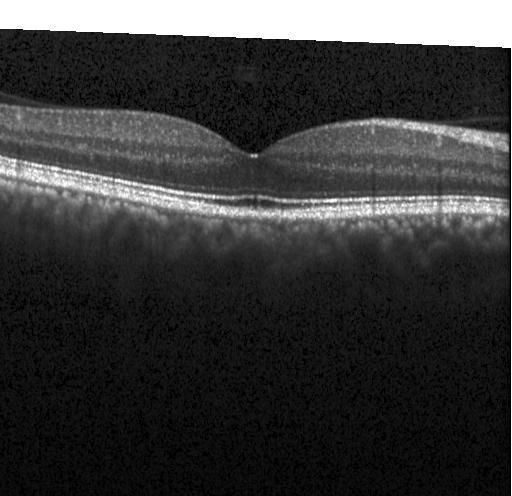 Spectral-domain optical coherence tomography. Retinal OCT cross-section.
Impression: no CNV, no DME, and no drusen.